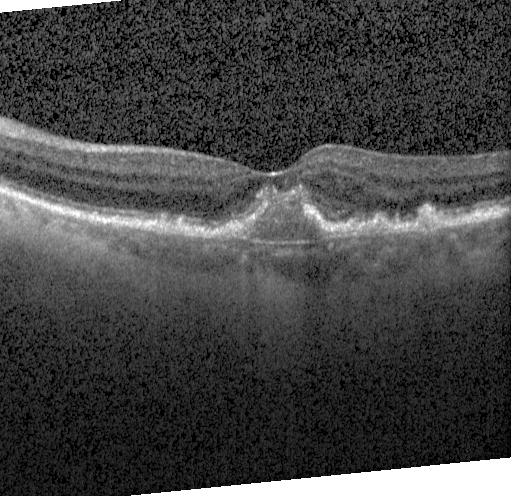

SD-OCT; Heidelberg Spectralis OCT system; OCT line scan. Impression: a choroidal neovascular membrane.